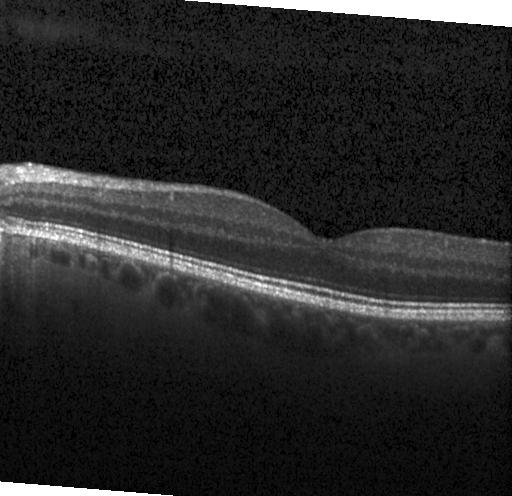
Macular scan. Retinal OCT B-scan. Finding: no CNV, DME, or drusen.